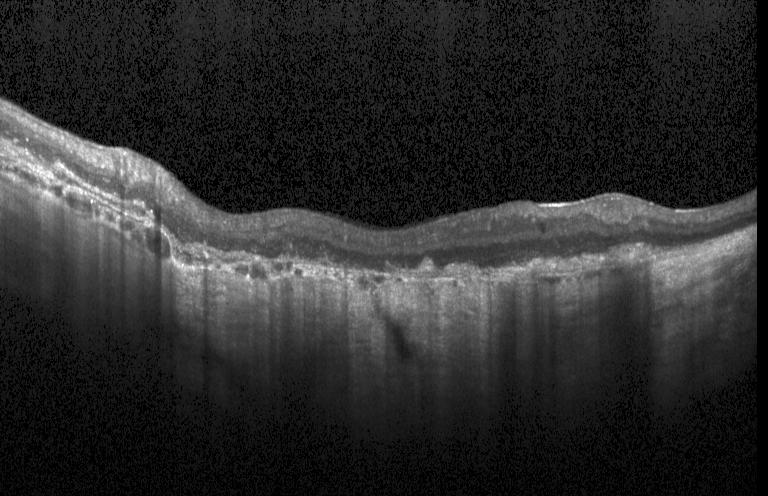 Retinal OCT cross-section · through the macula.
Impression: a choroidal neovascular membrane.